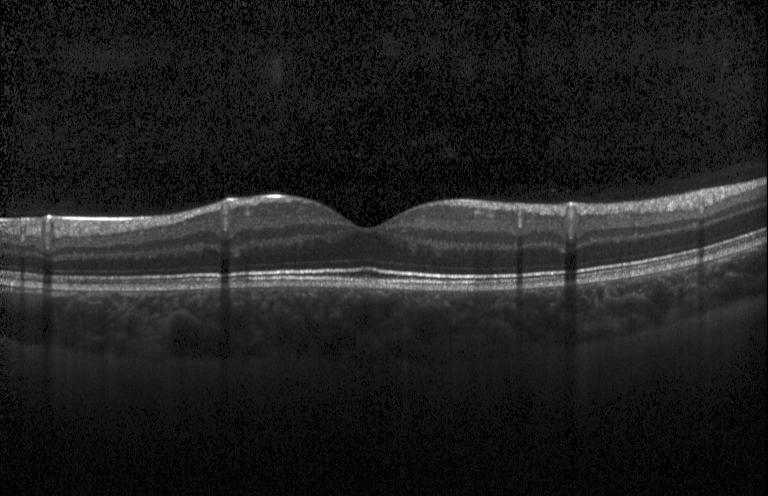 OCT B-scan. Dx: neither choroidal neovascularization, diabetic macular edema, nor drusen.